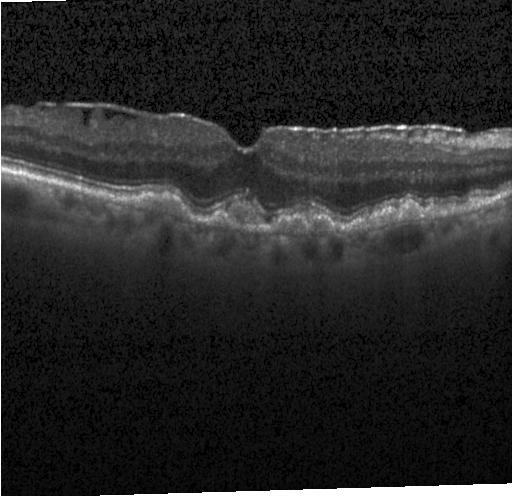
OCT B-scan. The scan shows sub-RPE drusenoid deposits.